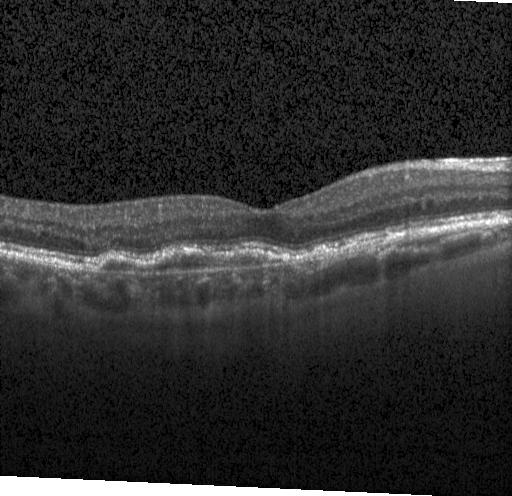

OCT line scan. Acquired on a Heidelberg Spectralis. Through the macula. Spectral-domain optical coherence tomography. Diagnosis: choroidal neovascularization (CNV).